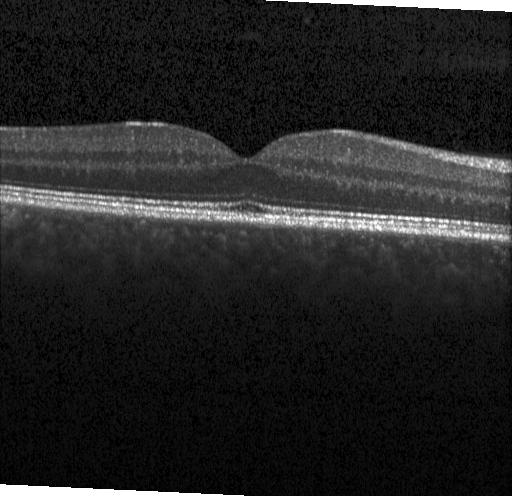 Centered on the fovea, OCT line scan, instrument: Heidelberg Spectralis — The scan shows no choroidal neovascularization, no diabetic macular edema, and no drusen.